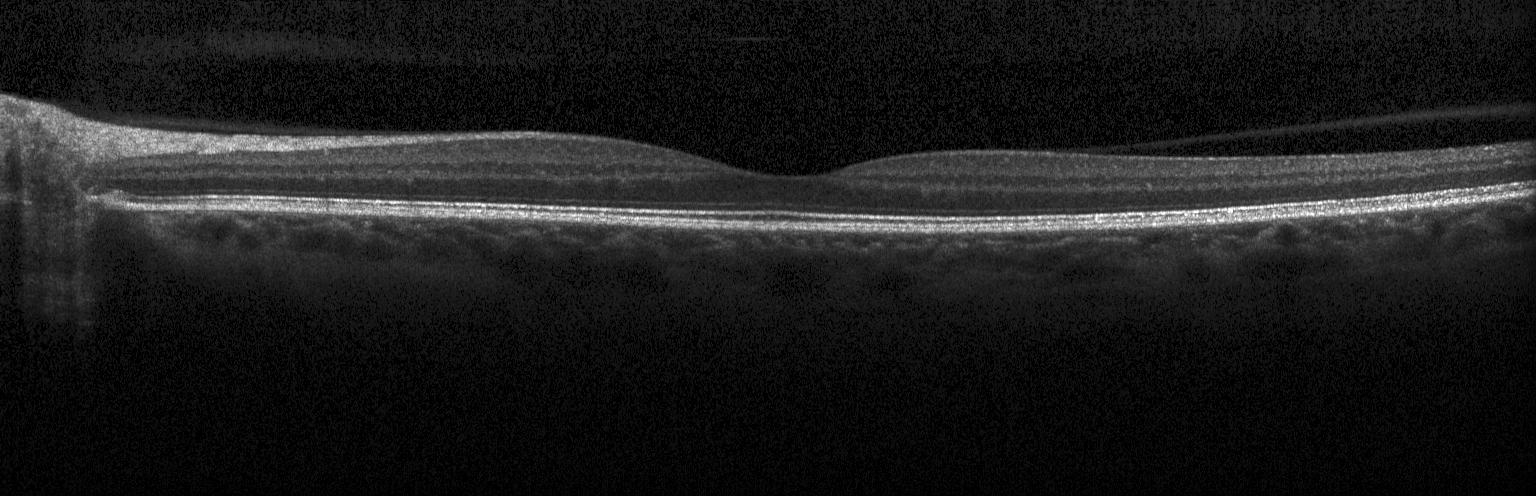 Macular OCT: no evidence of choroidal neovascularization, diabetic macular edema, or drusen.